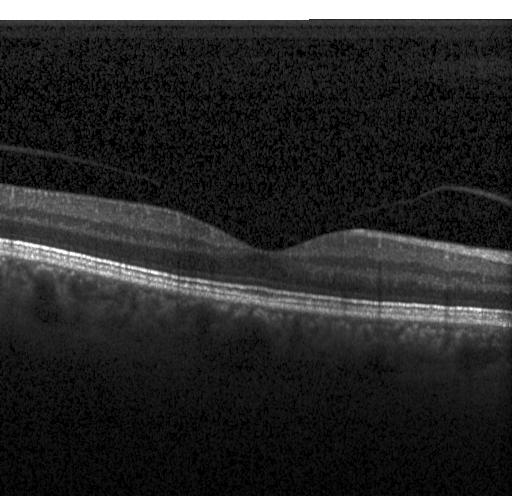
SD-OCT; OCT line scan; Heidelberg Spectralis OCT system — OCT finding: neither choroidal neovascularization, diabetic macular edema, nor drusen.